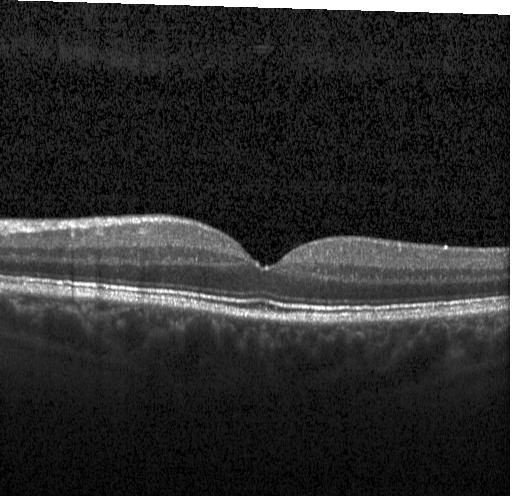

Impression: no choroidal neovascularization, diabetic macular edema, or drusen.